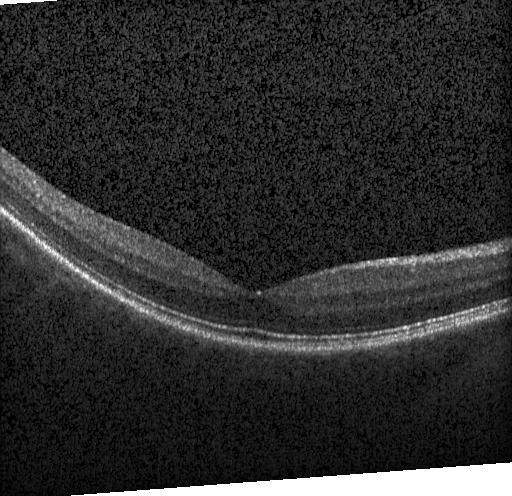

No CNV, no DME, and no drusen.